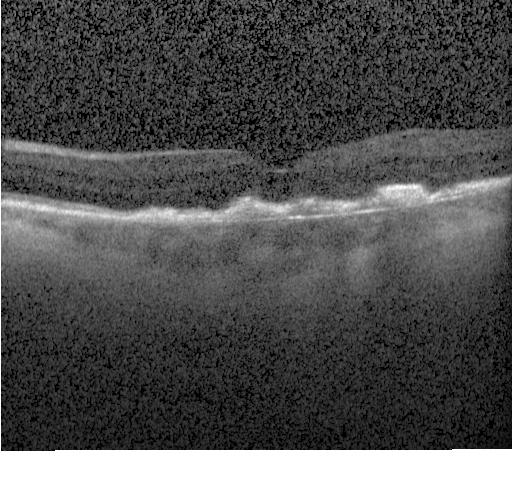

Finding: a choroidal neovascular membrane.